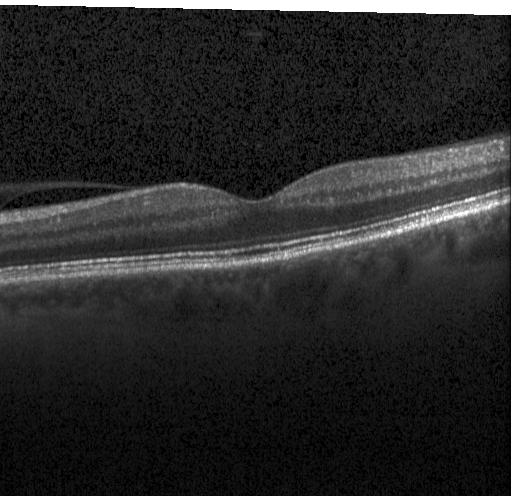
Optical coherence tomography B-scan, acquired on a Heidelberg Spectralis, through the macula.
Finding: no choroidal neovascularization, no diabetic macular edema, and no drusen.